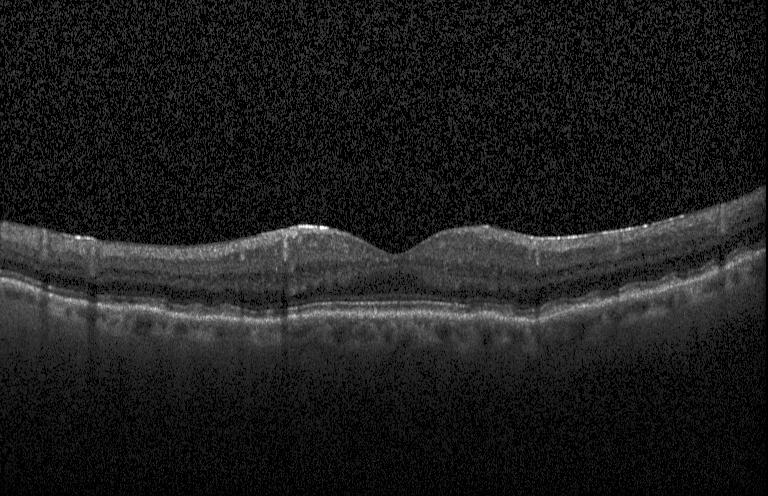 Finding: multiple drusen.